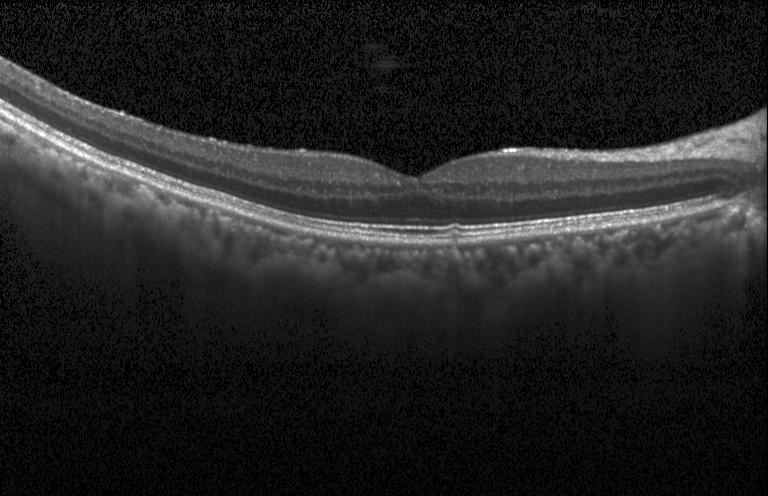 Spectral-domain optical coherence tomography. Acquired on a Heidelberg Spectralis. Retinal OCT cross-section. Fovea-centered
Finding: no CNV, no DME, and no drusen.